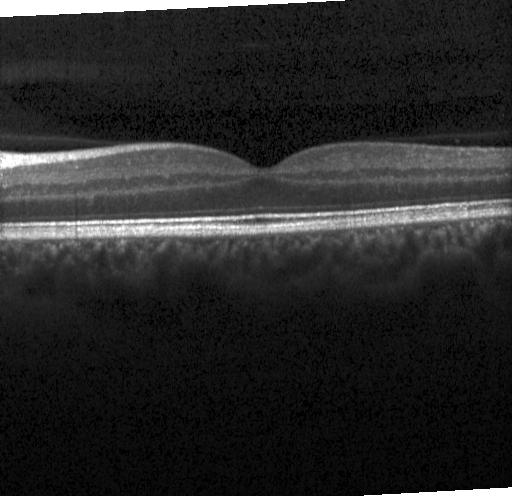
OCT line scan. Impression: no choroidal neovascularization, diabetic macular edema, or drusen.